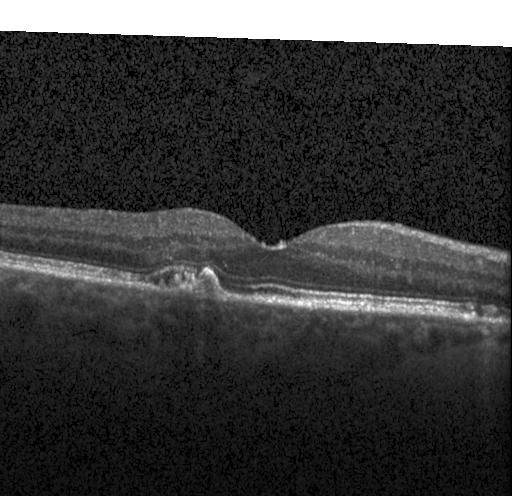

The scan shows a choroidal neovascular membrane.